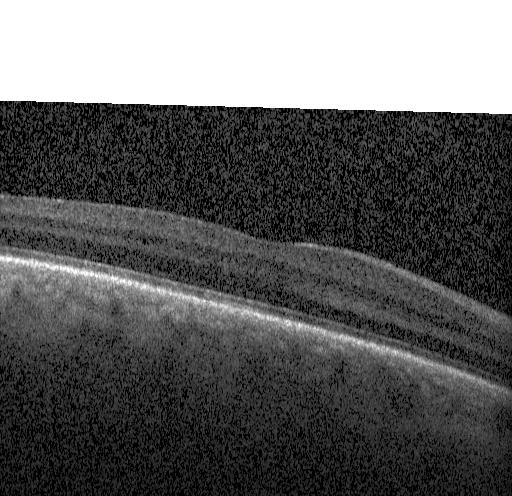

Optical coherence tomography scan, fovea-centered.
Finding: no evidence of choroidal neovascularization, diabetic macular edema, or drusen.